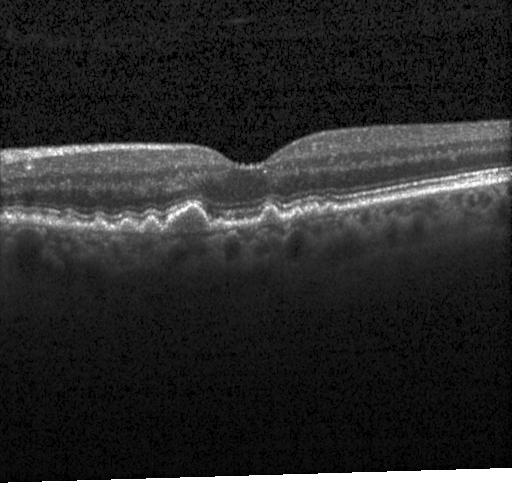

Sub-RPE drusenoid deposits.